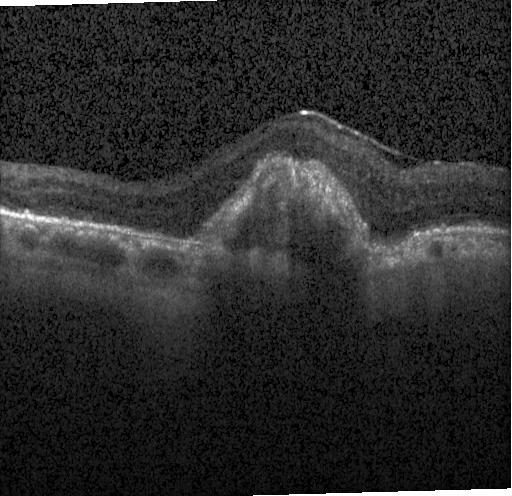 OCT finding: choroidal neovascularization (CNV).